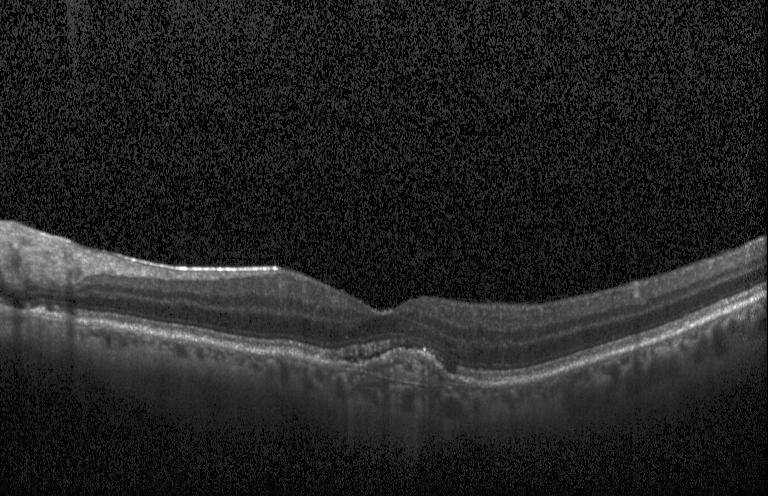 Optical coherence tomography scan
This B-scan demonstrates CNV.